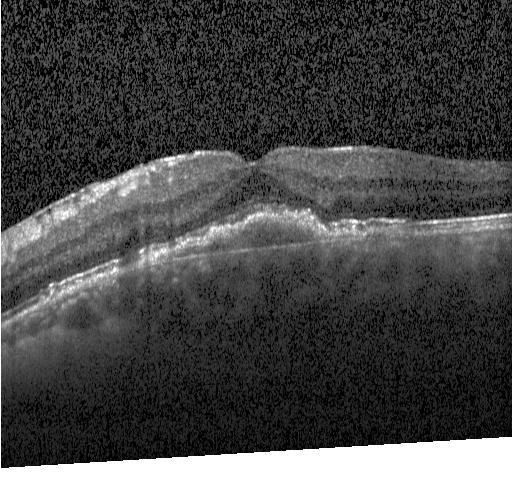 OCT B-scan; acquired on a Heidelberg Spectralis
Finding: a choroidal neovascular membrane.